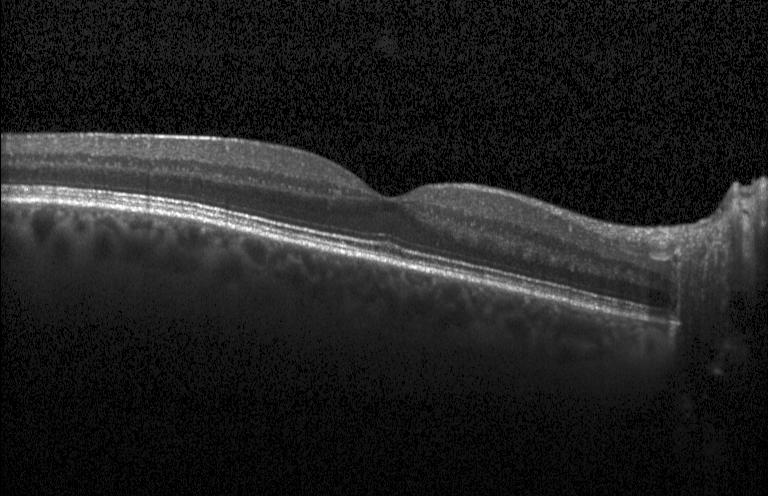

Retinal OCT B-scan
Finding: neither choroidal neovascularization, diabetic macular edema, nor drusen.